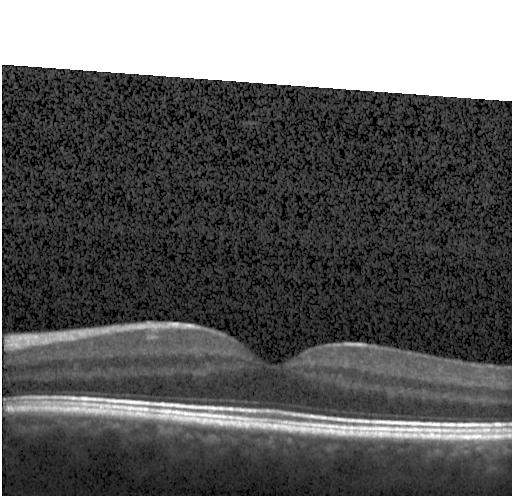

Finding: neither CNV, DME, nor drusen.